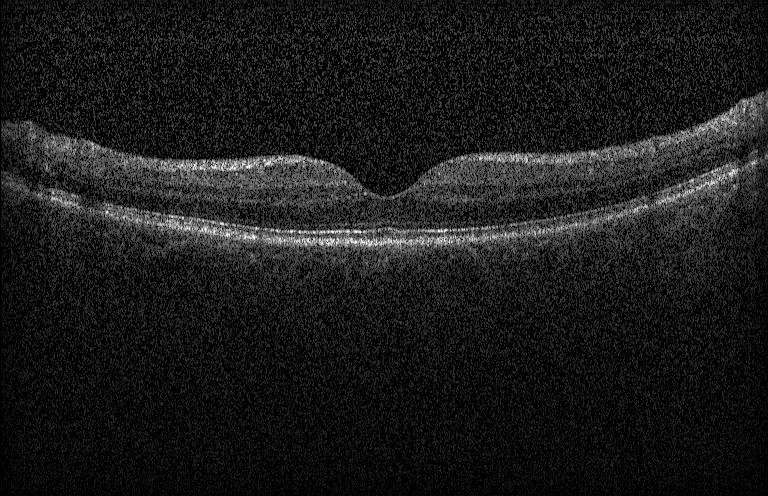

Retinal OCT B-scan — Diagnosis: no evidence of choroidal neovascularization, diabetic macular edema, or drusen.